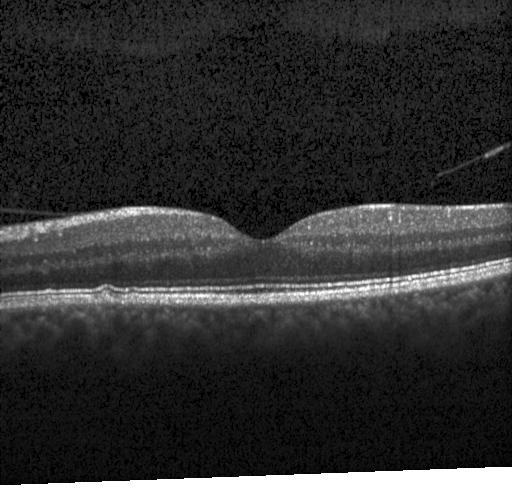

Dx: neither CNV, DME, nor drusen.